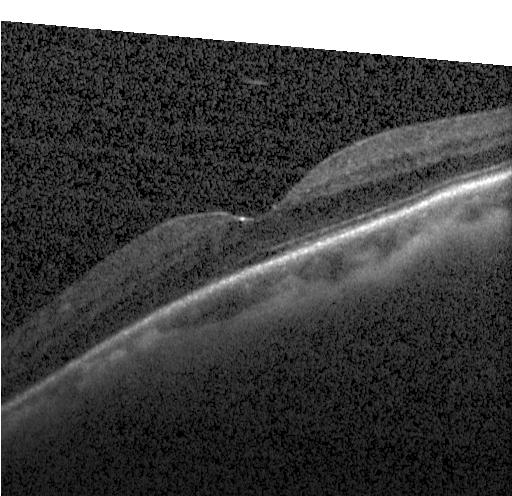 Retinal OCT cross-section — Diagnosis: no CNV, DME, or drusen.